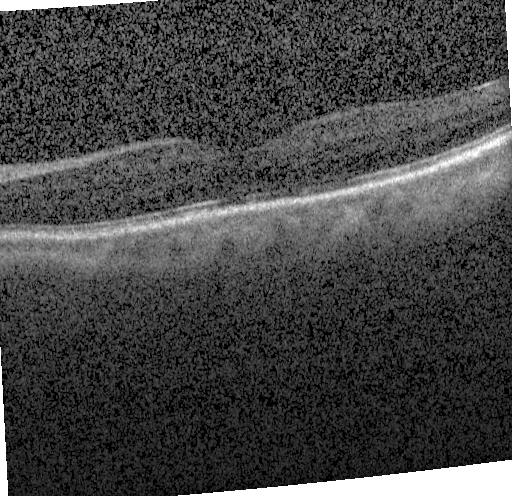
OCT line scan · spectral-domain optical coherence tomography · Heidelberg Spectralis OCT system · macular scan
Macular OCT: no choroidal neovascularization, no diabetic macular edema, and no drusen.